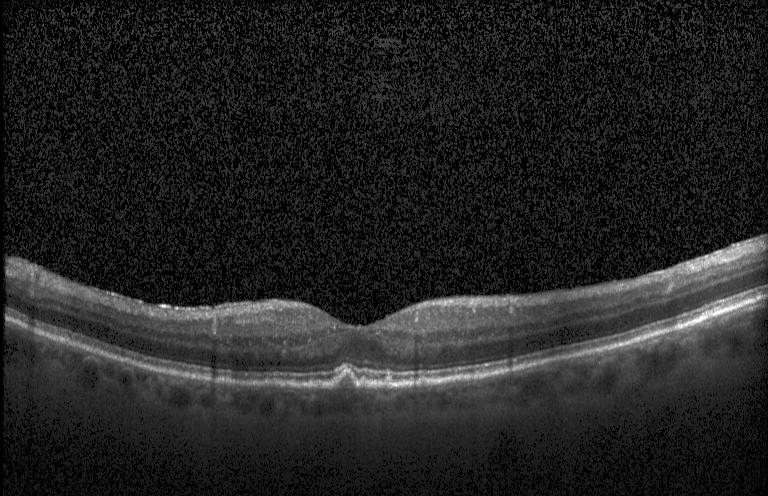 Impression: multiple drusen.